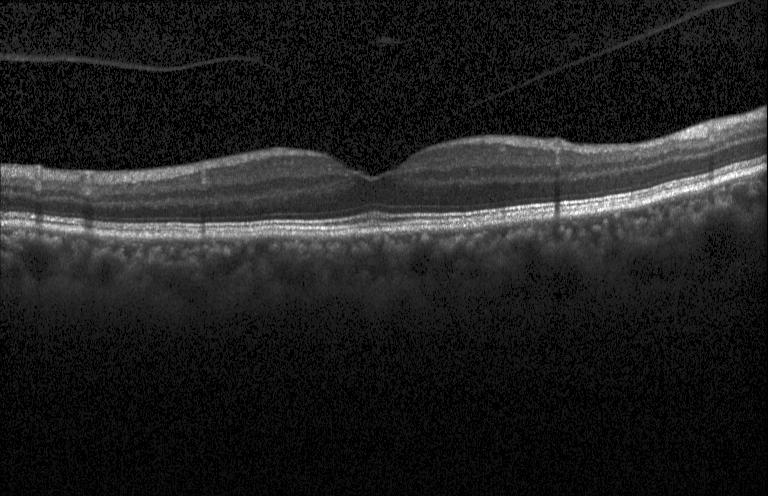
Macular OCT demonstrating no choroidal neovascularization, diabetic macular edema, or drusen.